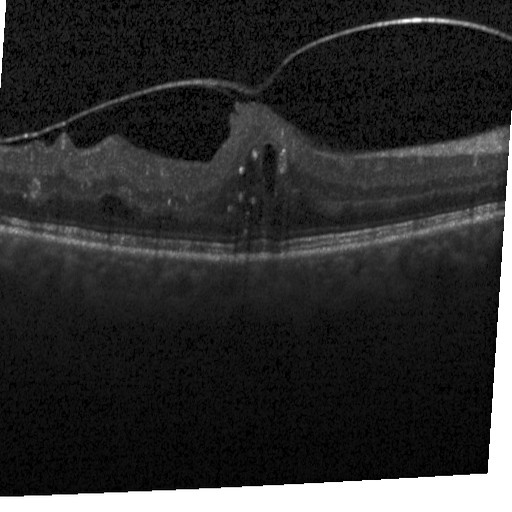 Retinal OCT cross-section. SD-OCT. Fovea-centered. Assessment: DME.